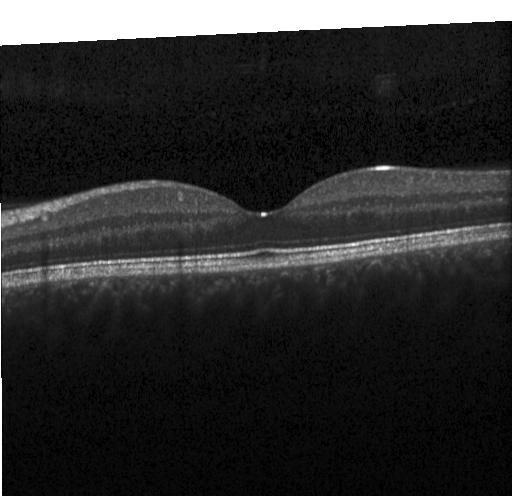
Fovea-centered. Heidelberg Spectralis. Retinal OCT cross-section.
No choroidal neovascularization, diabetic macular edema, or drusen.